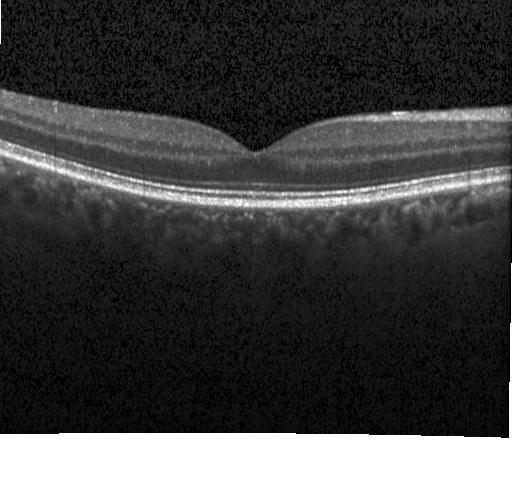 Finding: no evidence of CNV, DME, or drusen.